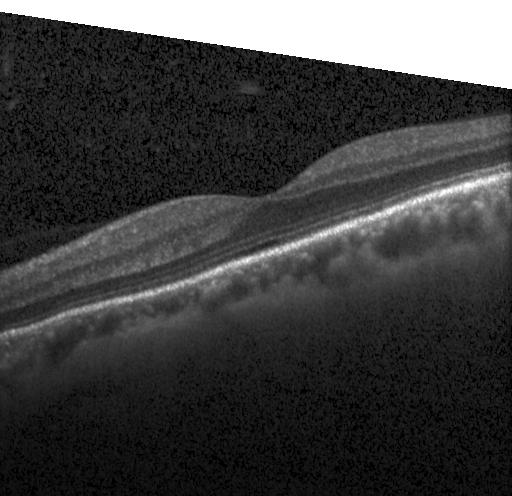 Centered on the fovea, OCT B-scan, SD-OCT. Finding: no evidence of CNV, DME, or drusen.